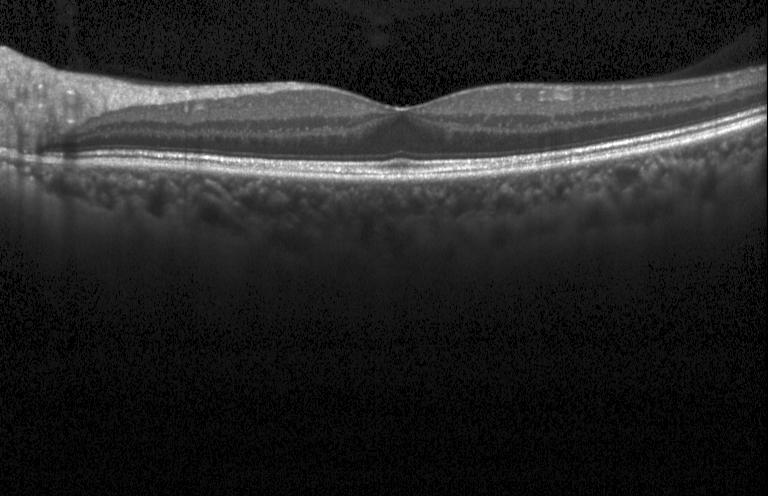

OCT finding: no choroidal neovascularization, diabetic macular edema, or drusen.